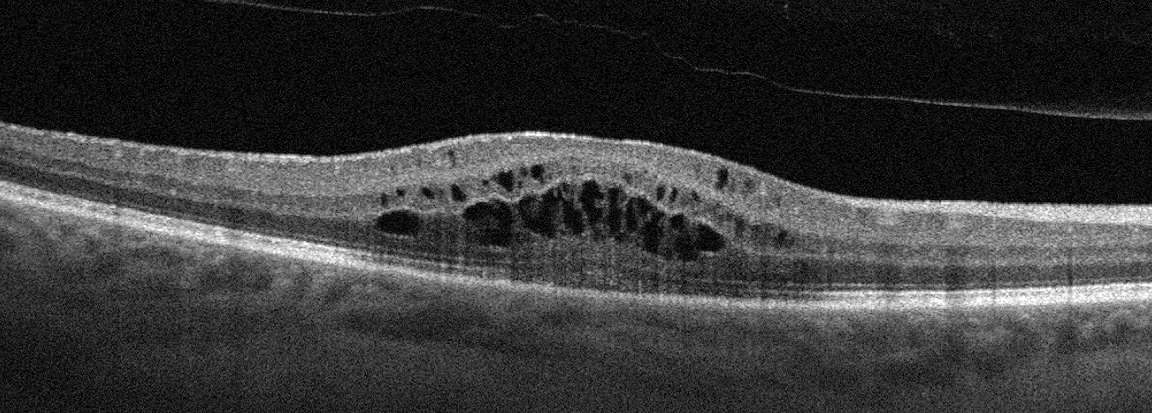

Through the macula; optical coherence tomography scan
Diagnosis: DME.